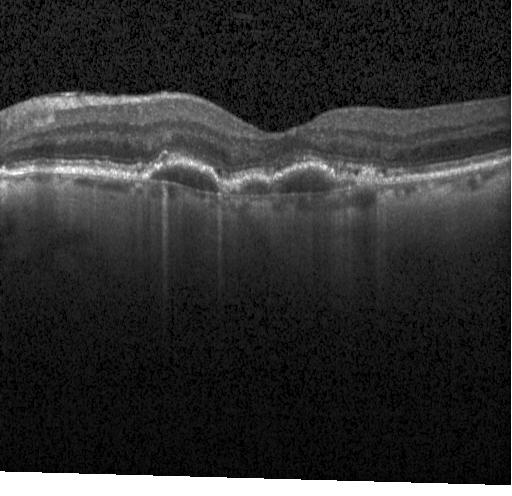

Spectral-domain optical coherence tomography. Retinal OCT cross-section
Diagnosis: a choroidal neovascular membrane.